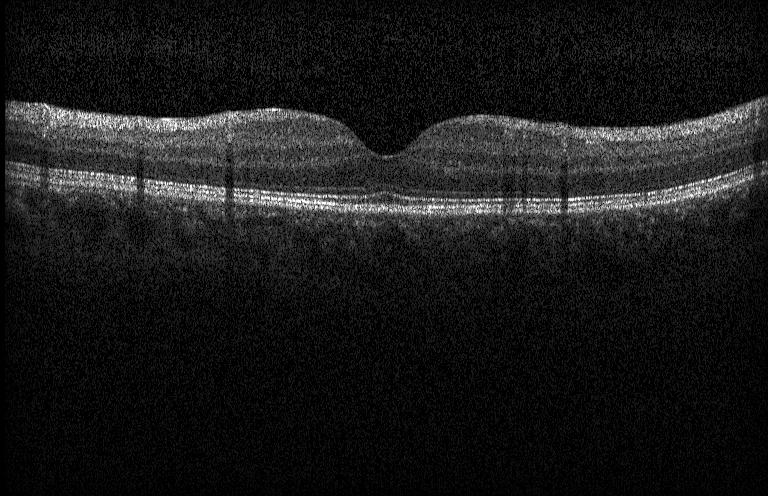
Acquired on a Heidelberg Spectralis; optical coherence tomography B-scan; SD-OCT; through the macula.
This B-scan demonstrates no choroidal neovascularization, diabetic macular edema, or drusen.